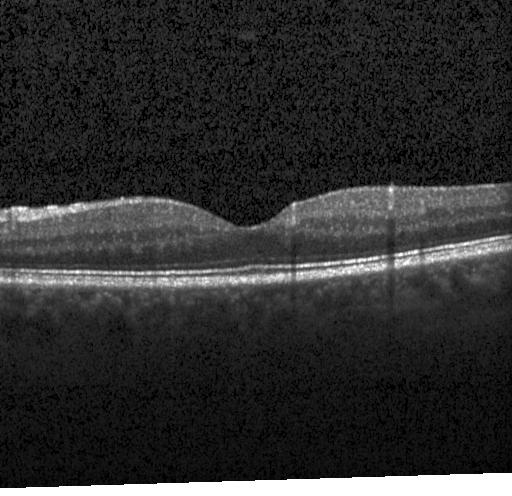 OCT finding: no evidence of choroidal neovascularization, diabetic macular edema, or drusen.